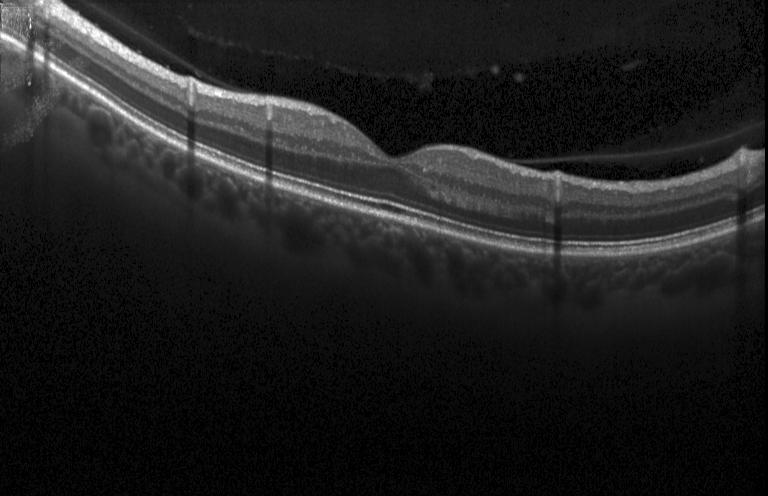
SD-OCT; retinal OCT B-scan.
Finding: no CNV, no DME, and no drusen.